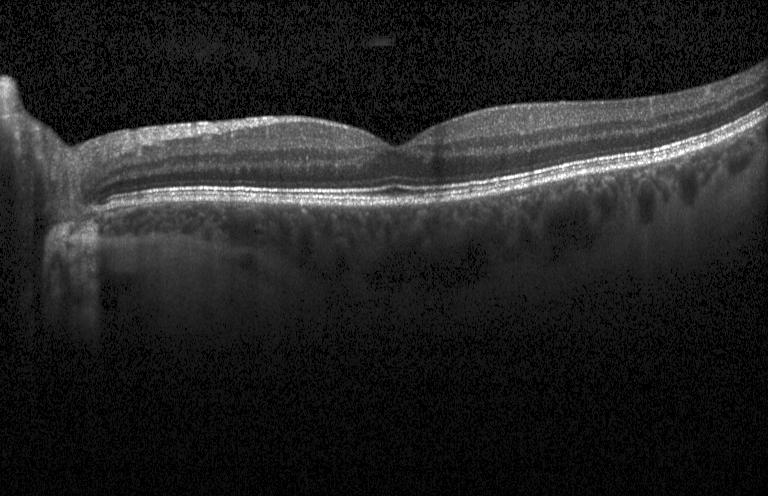 Macular OCT demonstrating no evidence of choroidal neovascularization, diabetic macular edema, or drusen.